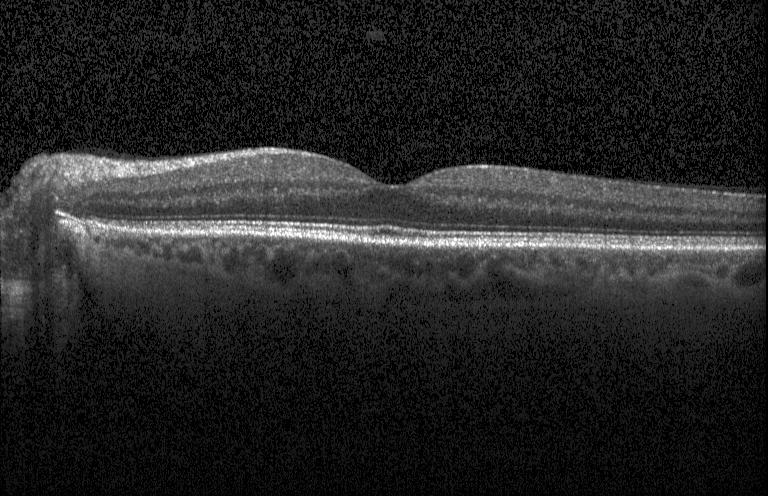
Assessment: no CNV, DME, or drusen.